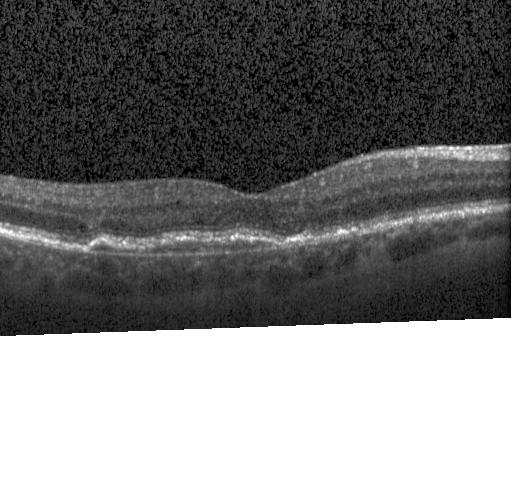 A choroidal neovascular membrane.